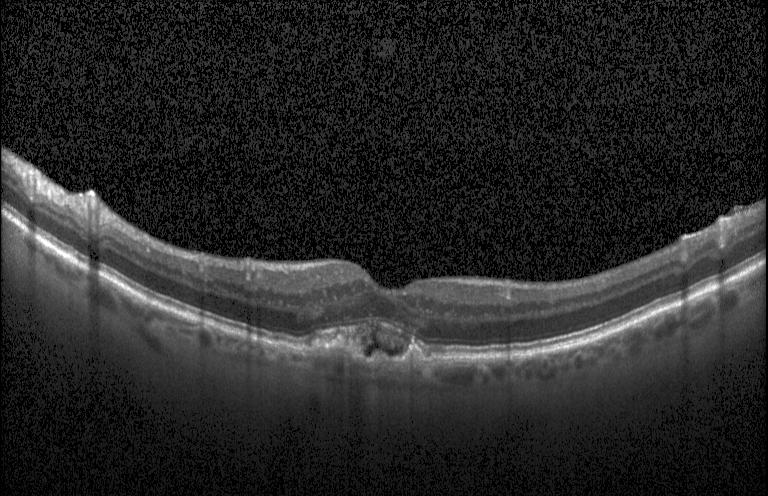 Horizontal scan through the fovea. SD-OCT. Heidelberg Spectralis OCT system. Optical coherence tomography scan
Impression: a choroidal neovascular membrane.